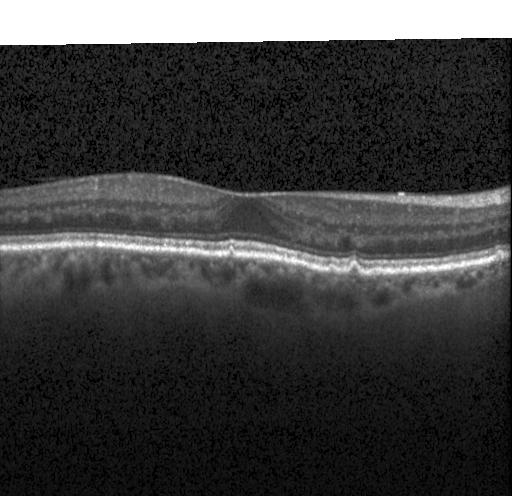

Dx: drusen.